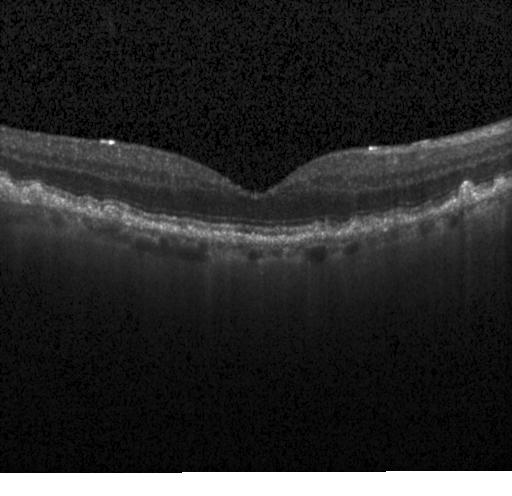
Acquired on a Heidelberg Spectralis, OCT B-scan — Dx: sub-RPE drusenoid deposits.